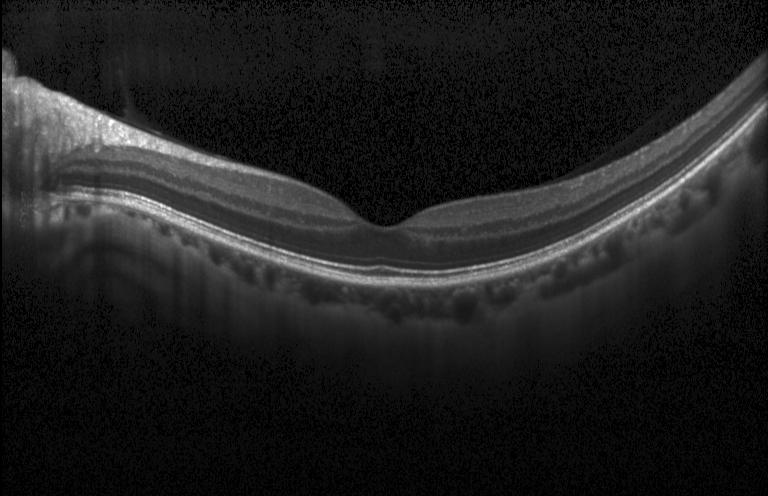 OCT B-scan; spectral-domain OCT; centered on the fovea; Heidelberg Spectralis OCT system — No choroidal neovascularization, diabetic macular edema, or drusen.